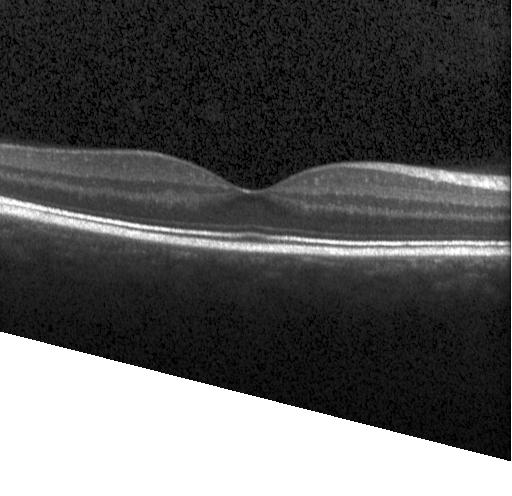 Retinal OCT cross-section. Macular OCT: no evidence of choroidal neovascularization, diabetic macular edema, or drusen.